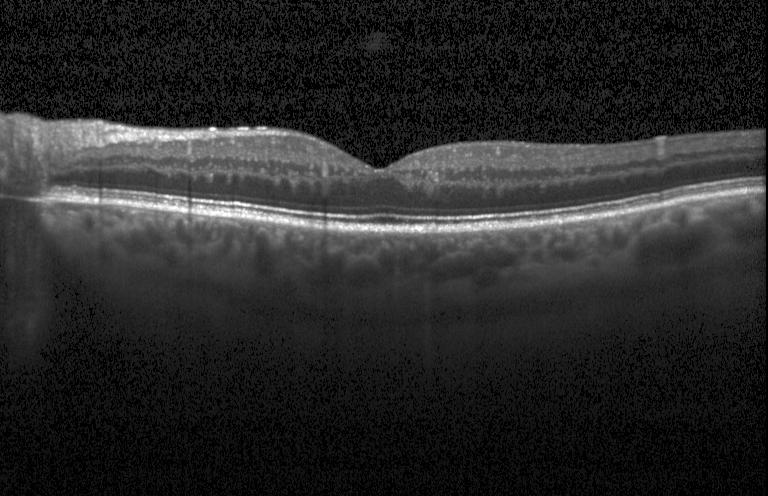 Dx: neither choroidal neovascularization, diabetic macular edema, nor drusen.